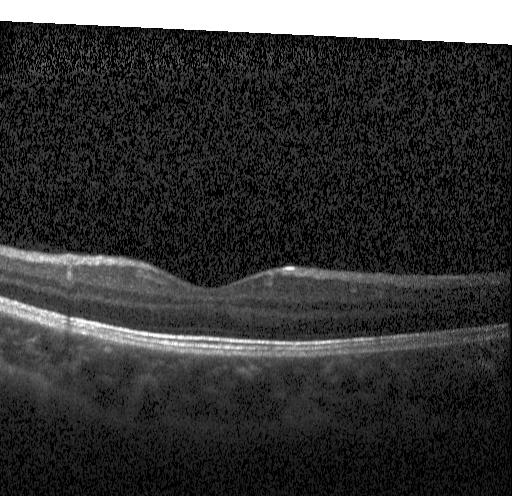

Finding: no choroidal neovascularization, diabetic macular edema, or drusen.